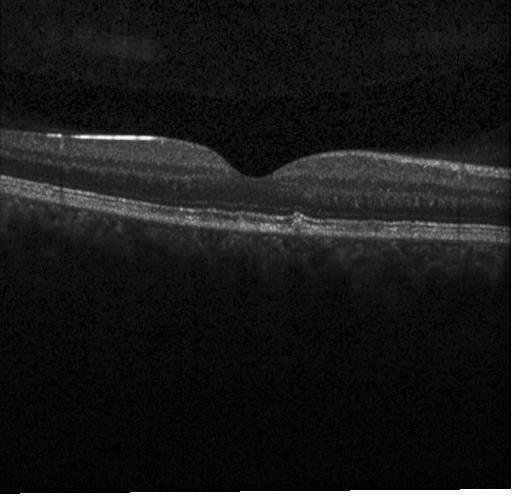
Dx: drusen.